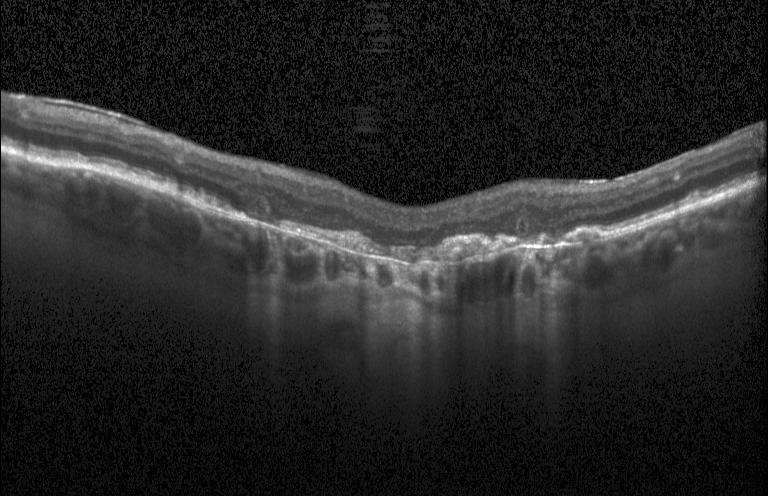

OCT B-scan; fovea-centered; SD-OCT — Impression: a choroidal neovascular membrane.